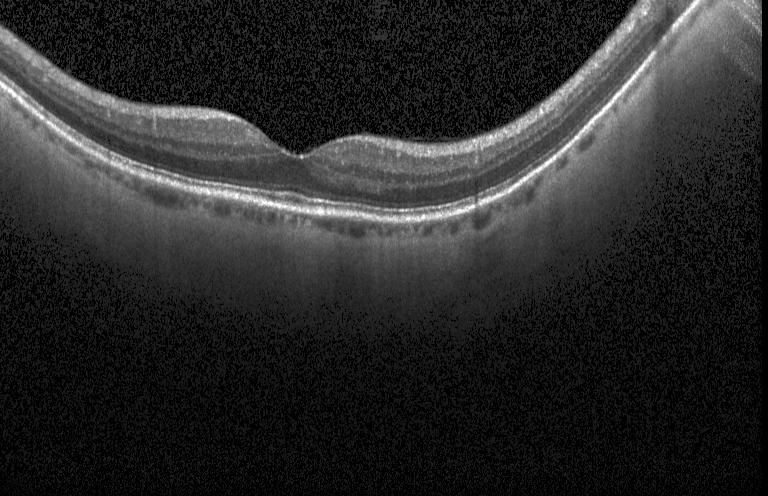
Optical coherence tomography B-scan — Finding: no choroidal neovascularization, no diabetic macular edema, and no drusen.